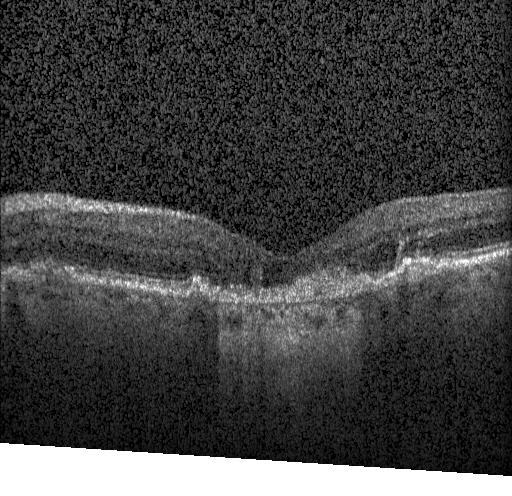 CNV.